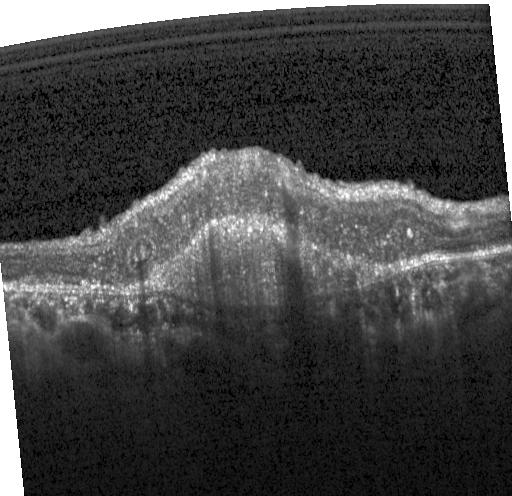
OCT line scan; SD-OCT; macular scan
Finding: choroidal neovascularization.